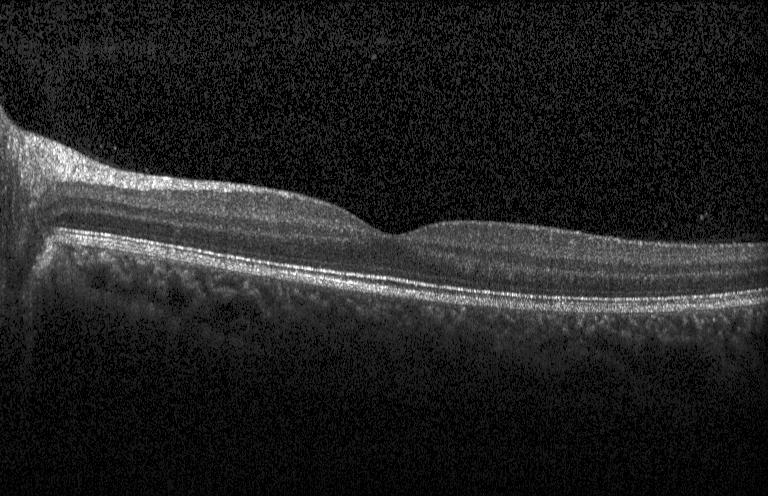 Impression: no CNV, DME, or drusen.